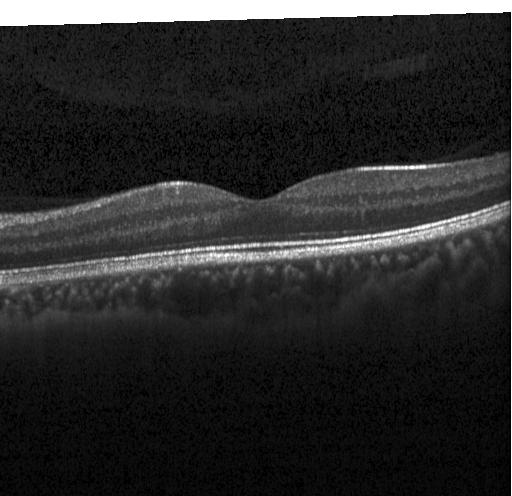 Neither choroidal neovascularization, diabetic macular edema, nor drusen.